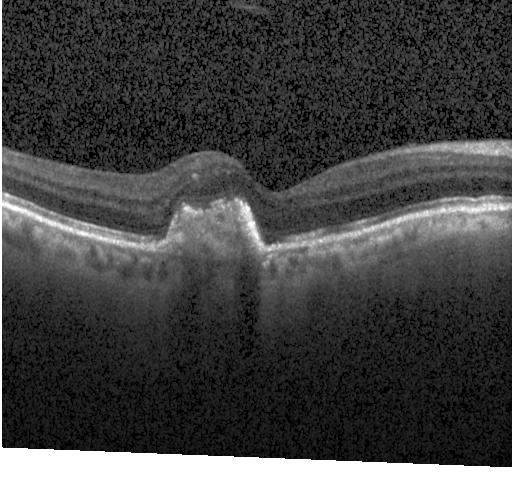 Horizontal scan through the fovea · SD-OCT · optical coherence tomography B-scan
Impression: choroidal neovascularization.